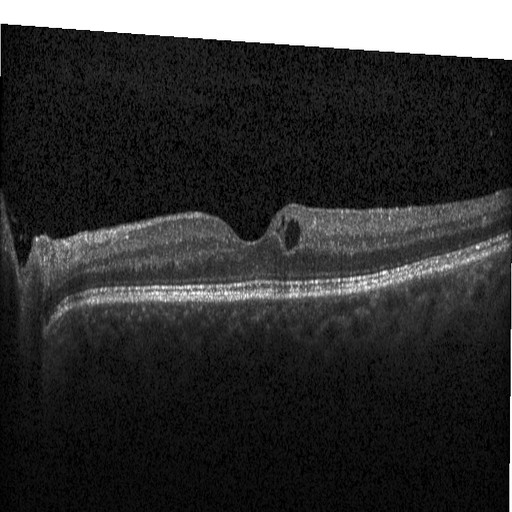 Impression: diabetic macular edema.